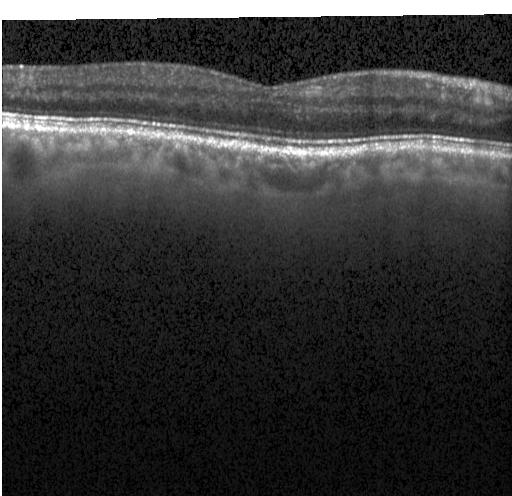
This B-scan demonstrates no choroidal neovascularization, no diabetic macular edema, and no drusen.